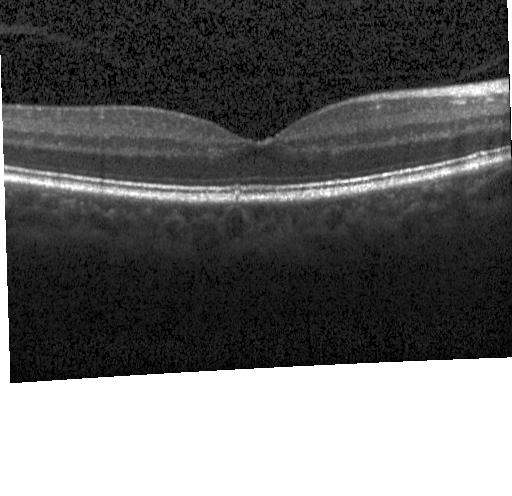 Instrument: Heidelberg Spectralis. Spectral-domain optical coherence tomography. Optical coherence tomography B-scan — Dx: drusen.